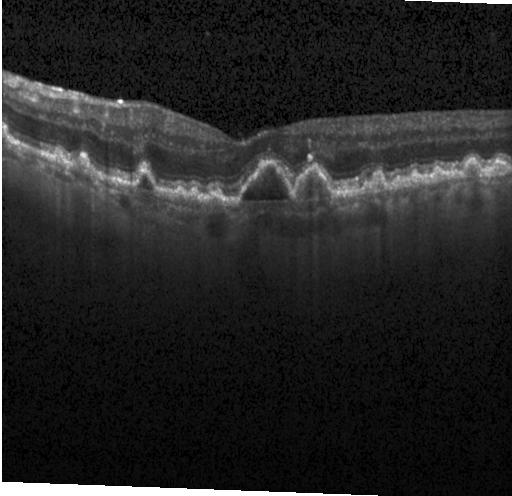 Retinal OCT cross-section, Heidelberg Spectralis OCT system, spectral-domain OCT — Assessment: sub-RPE drusenoid deposits.